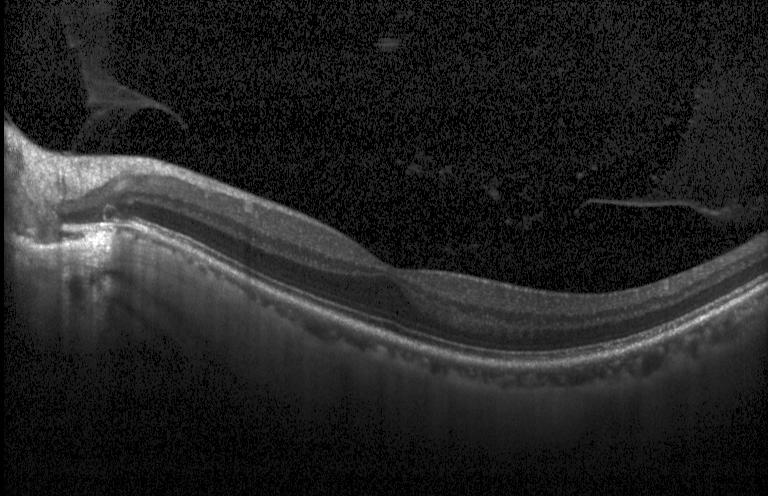
Optical coherence tomography scan; through the macula — Finding: no choroidal neovascularization, diabetic macular edema, or drusen.